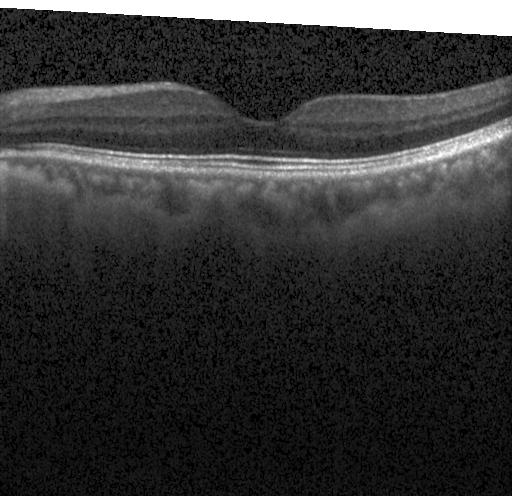

Macular OCT demonstrating neither choroidal neovascularization, diabetic macular edema, nor drusen.